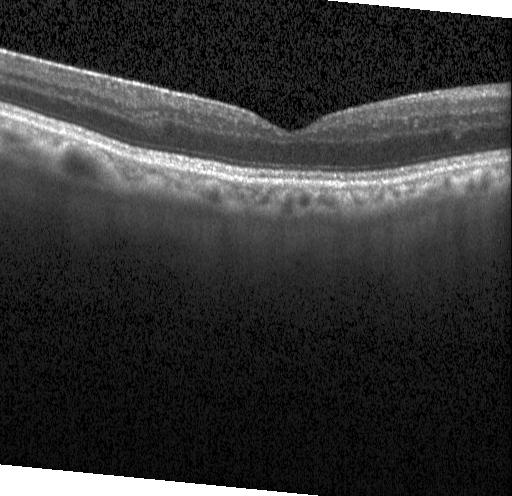 Assessment: no evidence of choroidal neovascularization, diabetic macular edema, or drusen.